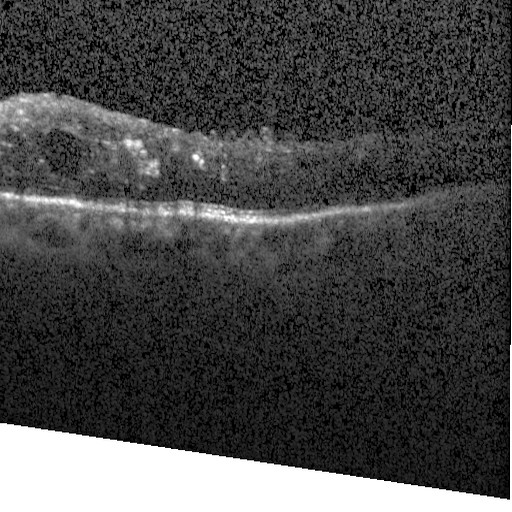

Fovea-centered. Heidelberg Spectralis OCT system. SD-OCT. Retinal OCT B-scan.
The scan shows diabetic macular edema (DME).